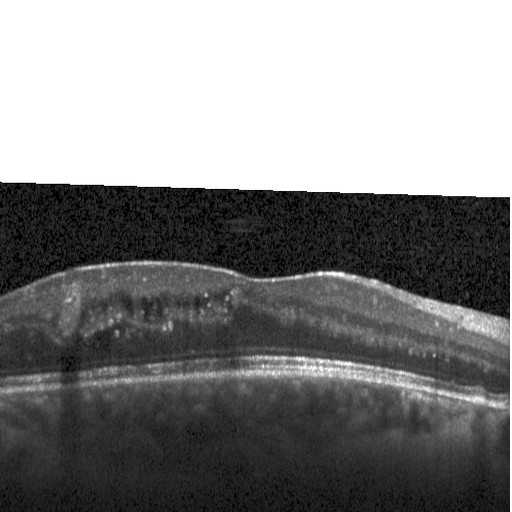

Macular OCT: DME.